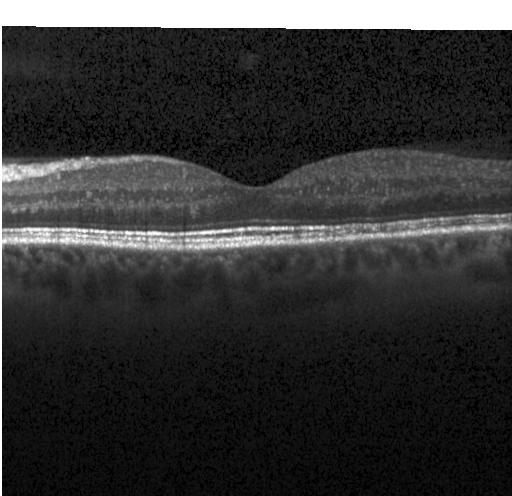
Optical coherence tomography scan, spectral-domain optical coherence tomography, acquired on a Heidelberg Spectralis — Impression: no choroidal neovascularization, diabetic macular edema, or drusen.